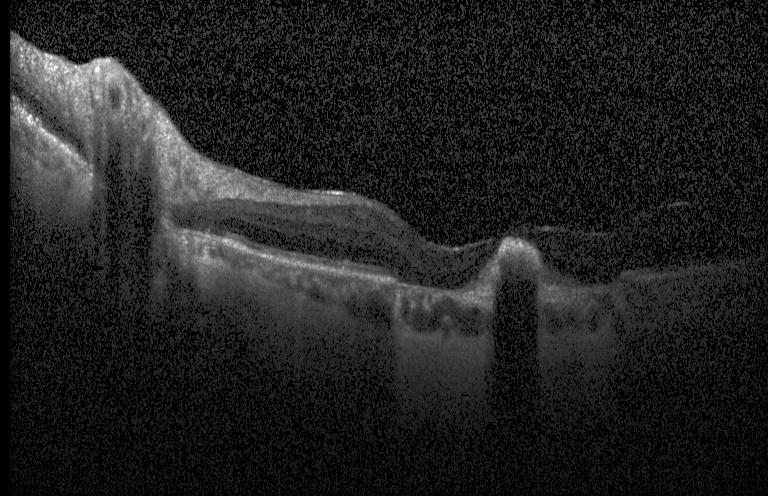
Optical coherence tomography B-scan
Macular OCT: a choroidal neovascular membrane.